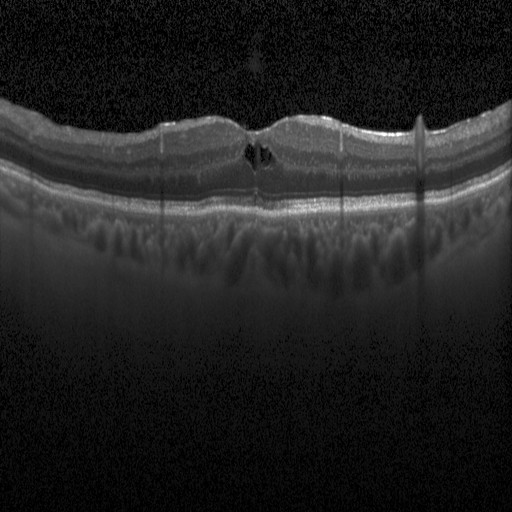 OCT B-scan — Finding: diabetic macular edema (DME).